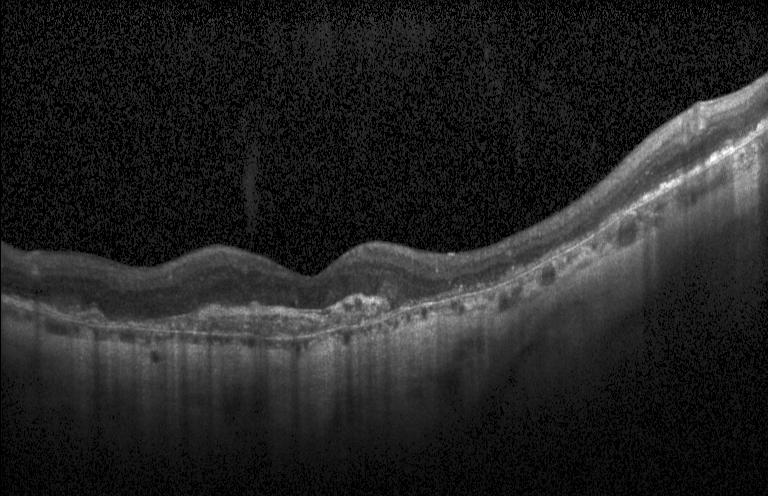

Impression: choroidal neovascularization (CNV).